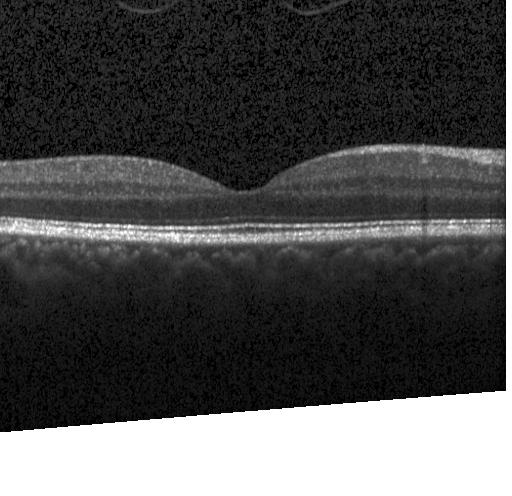
Retinal OCT B-scan; spectral-domain optical coherence tomography; fovea-centered; Heidelberg Spectralis.
Assessment: no CNV, DME, or drusen.